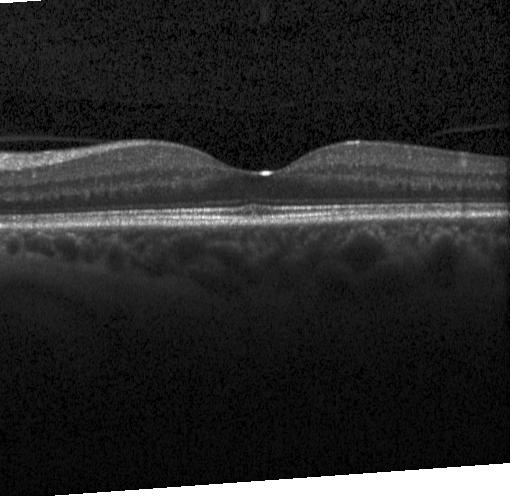 Retinal OCT B-scan · spectral-domain optical coherence tomography · Heidelberg Spectralis. Diagnosis: no evidence of choroidal neovascularization, diabetic macular edema, or drusen.